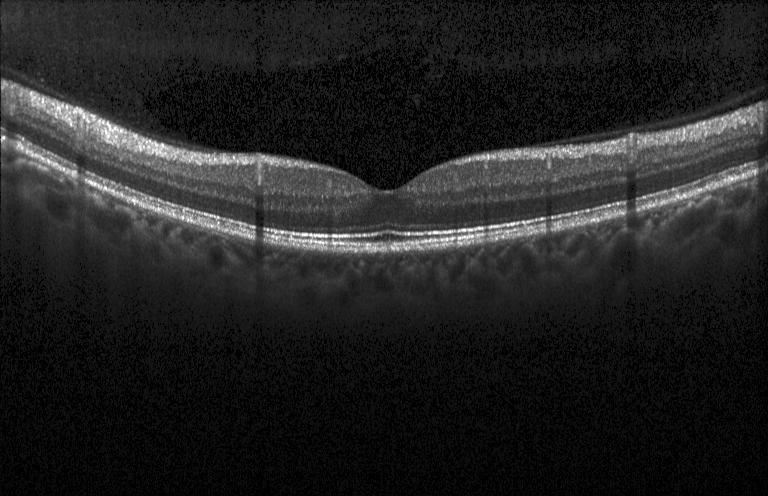 Diagnosis: no CNV, no DME, and no drusen.